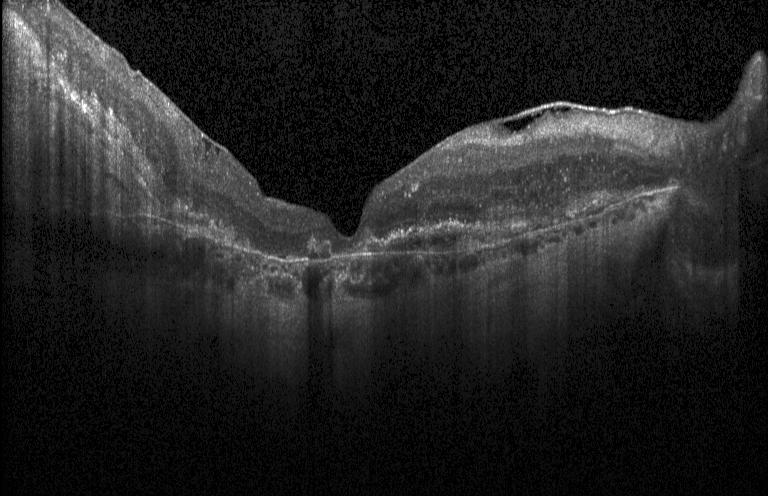 Fovea-centered, SD-OCT, retinal OCT B-scan.
Impression: a choroidal neovascular membrane.